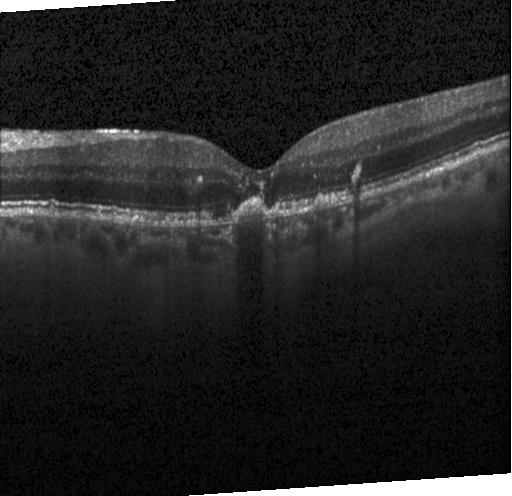

SD-OCT, retinal OCT B-scan, Heidelberg Spectralis. OCT finding: a choroidal neovascular membrane.